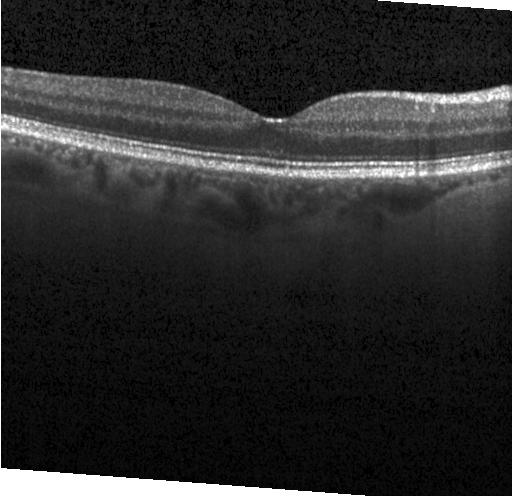

No evidence of choroidal neovascularization, diabetic macular edema, or drusen.